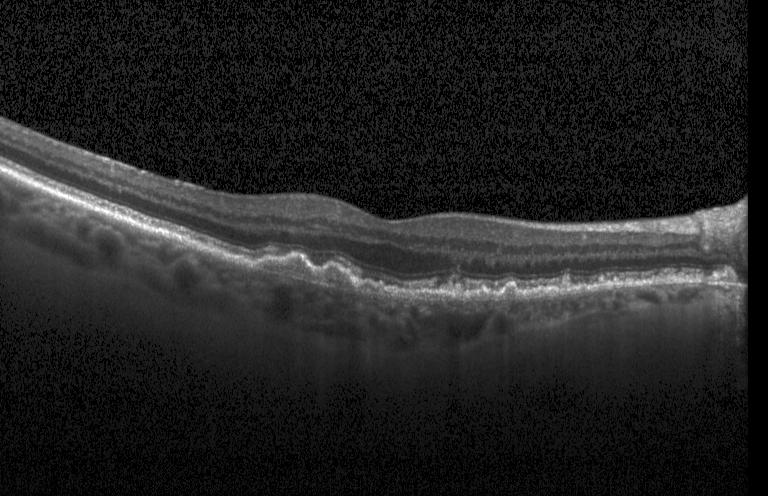 Acquired on a Heidelberg Spectralis, OCT line scan. Sub-RPE drusenoid deposits.